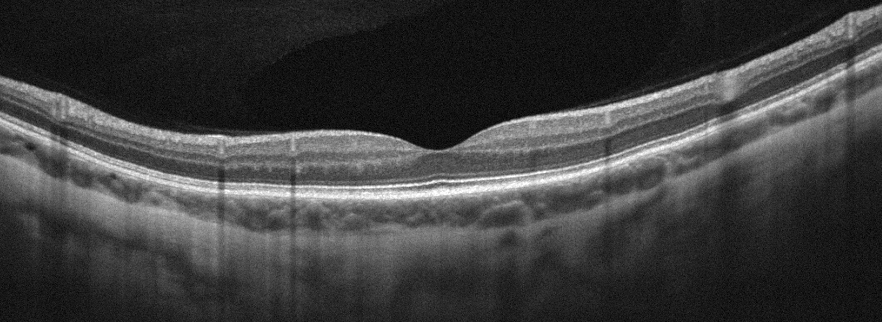
Diagnosis: no AMD, DME, ERM, RAO, RVO, or VID.